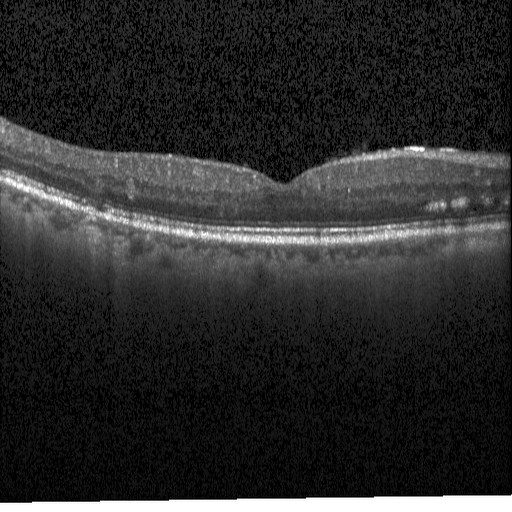 SD-OCT; optical coherence tomography scan.
Impression: DME.